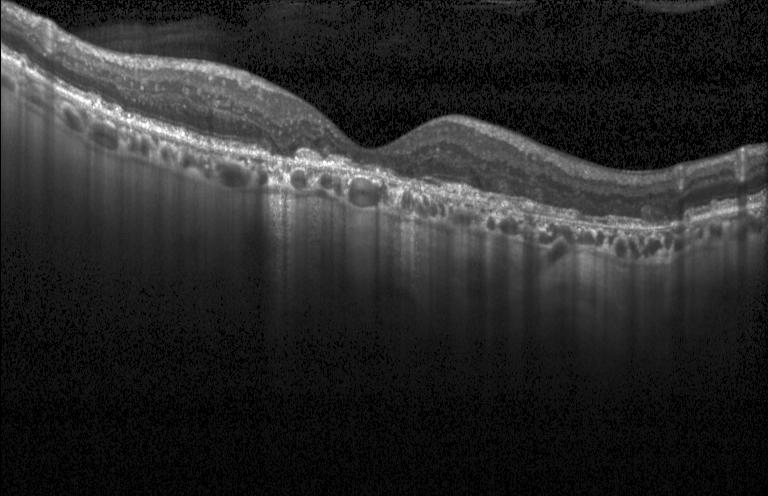
Diagnosis: choroidal neovascularization.